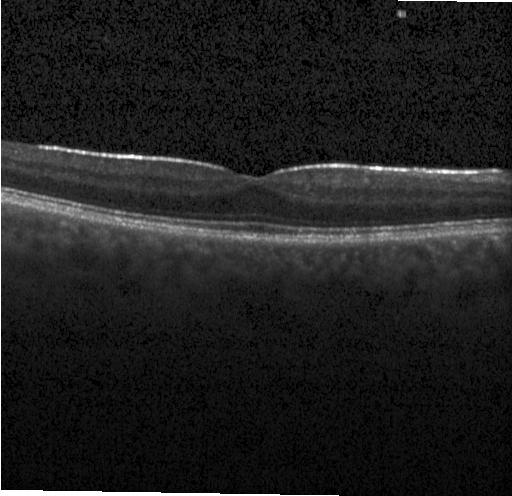

Centered on the fovea; OCT B-scan; acquired on a Heidelberg Spectralis.
Macular OCT: neither choroidal neovascularization, diabetic macular edema, nor drusen.